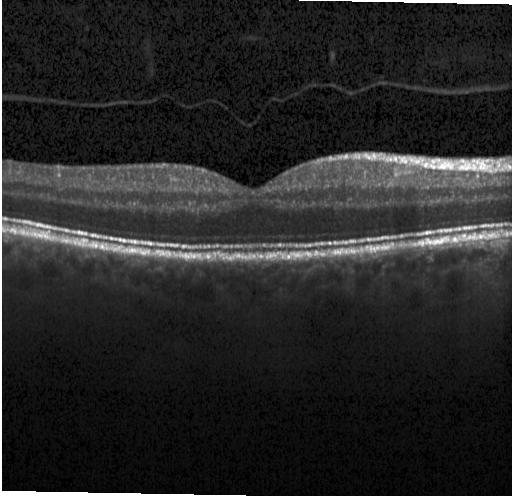 Retinal OCT cross-section; spectral-domain optical coherence tomography; acquired on a Heidelberg Spectralis; centered on the fovea. Assessment: neither choroidal neovascularization, diabetic macular edema, nor drusen.